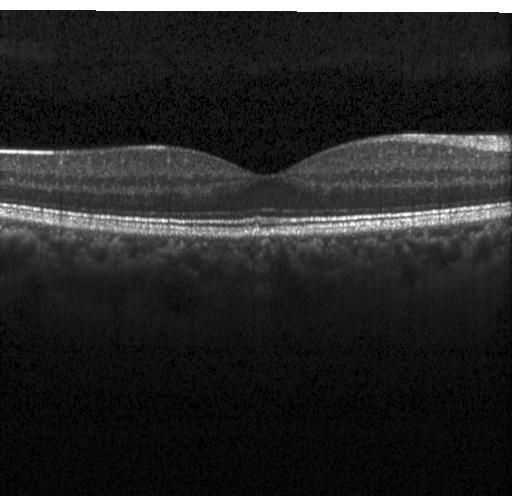
Dx: neither CNV, DME, nor drusen.